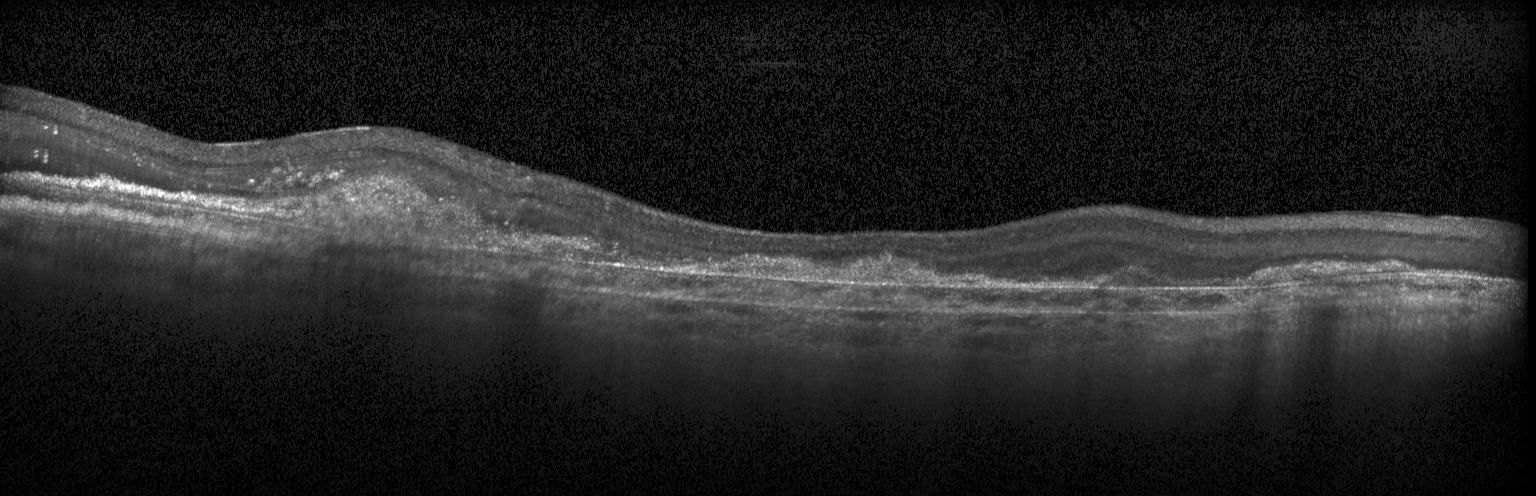 Diagnosis: a choroidal neovascular membrane.